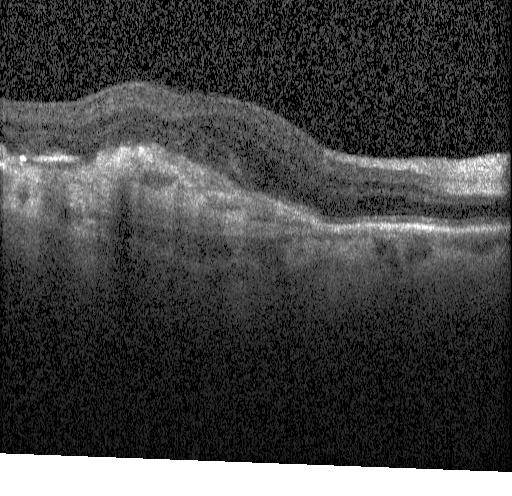

Retinal OCT B-scan — Finding: choroidal neovascularization.